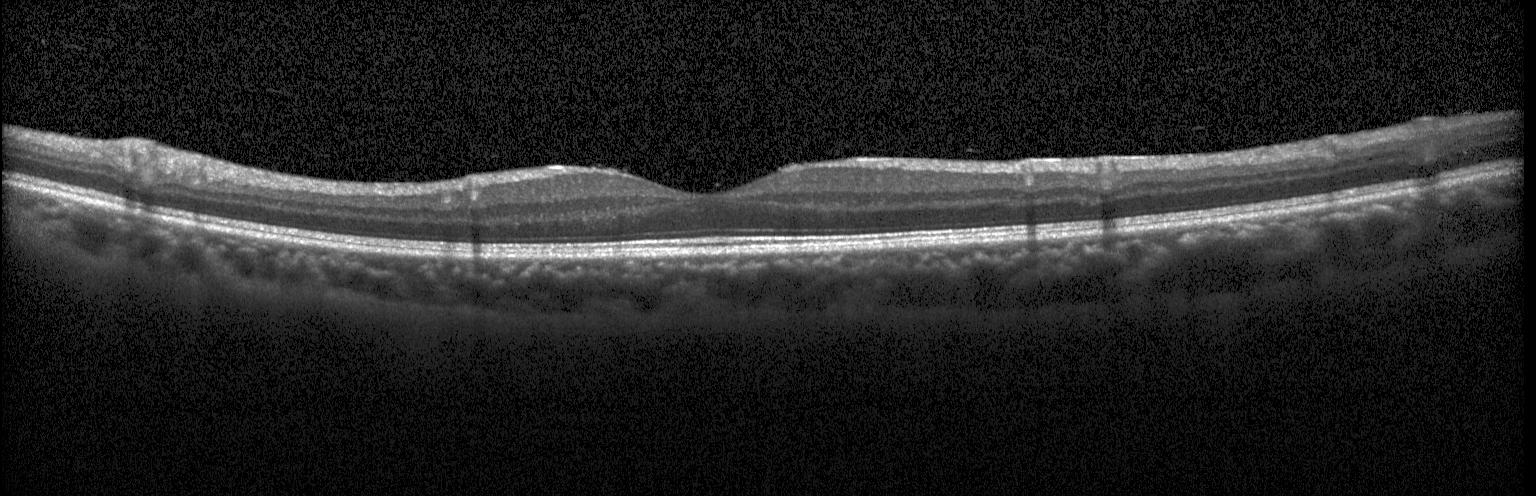

Spectral-domain OCT, optical coherence tomography scan — OCT finding: no evidence of choroidal neovascularization, diabetic macular edema, or drusen.